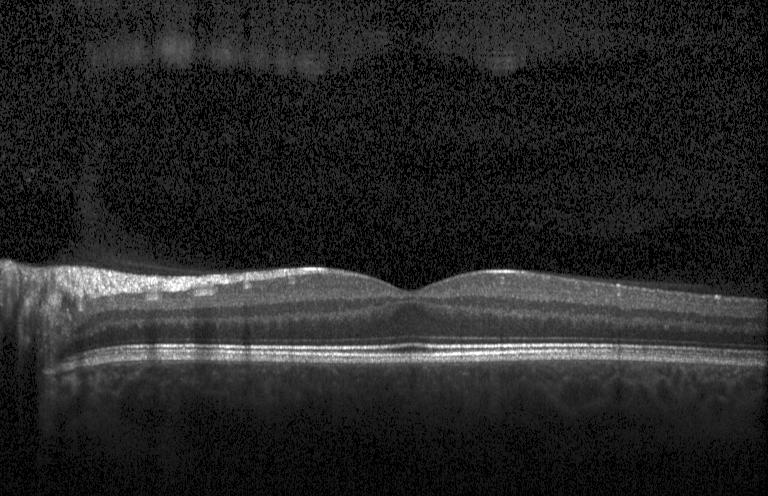

Impression: no CNV, no DME, and no drusen.